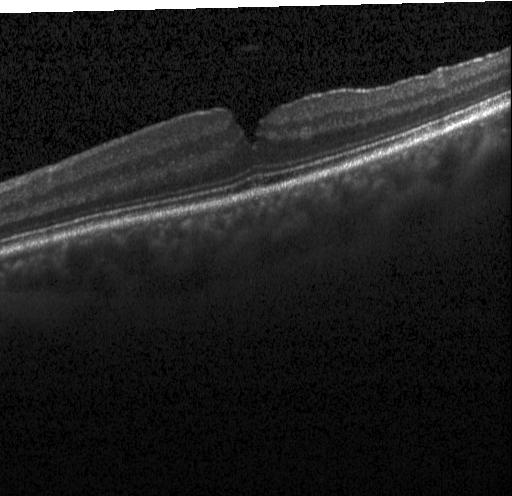

Finding: neither CNV, DME, nor drusen.